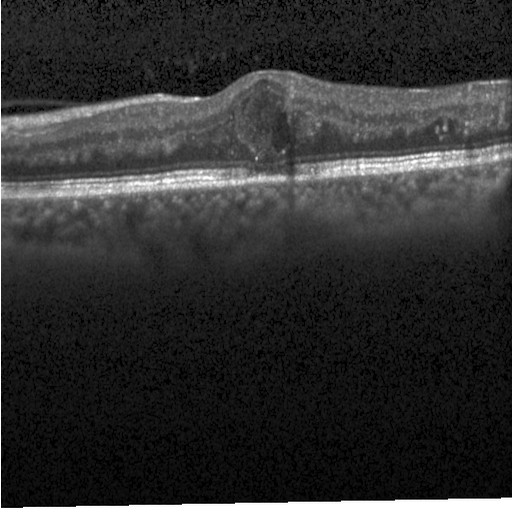

Assessment: diabetic macular edema (DME).